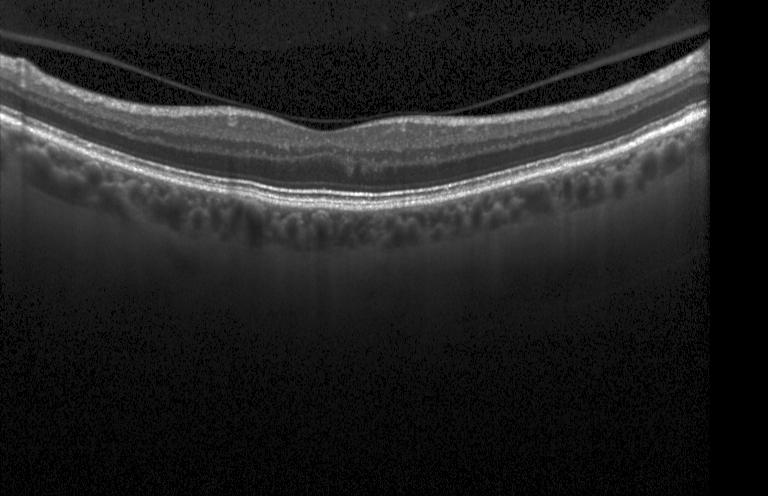 Assessment: neither choroidal neovascularization, diabetic macular edema, nor drusen.